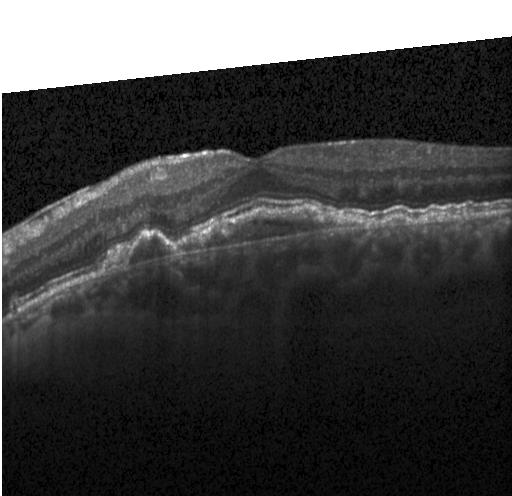

OCT B-scan
Assessment: a choroidal neovascular membrane.